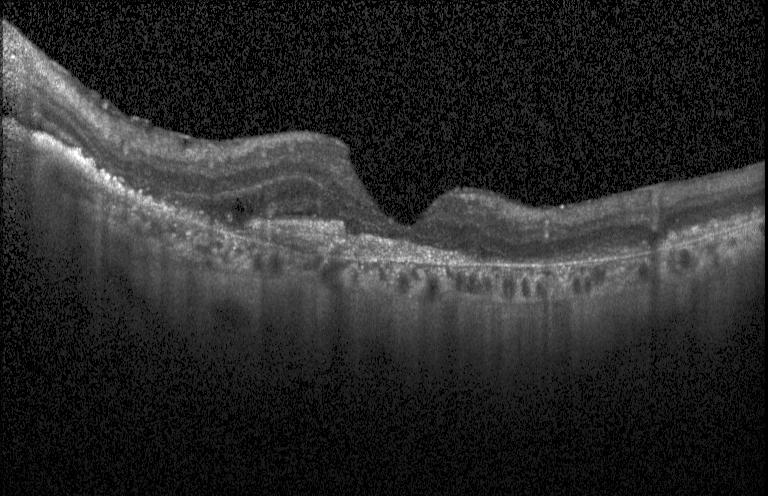 Optical coherence tomography B-scan; horizontal scan through the fovea.
Impression: a choroidal neovascular membrane.